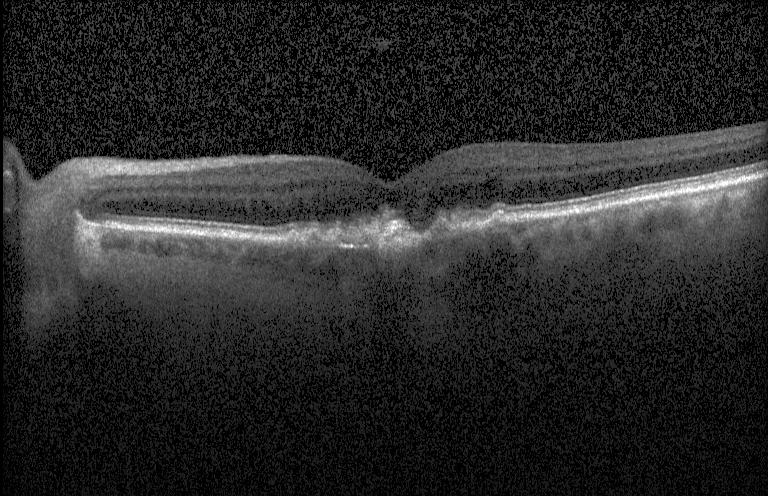

Retinal OCT B-scan
Finding: choroidal neovascularization (CNV).